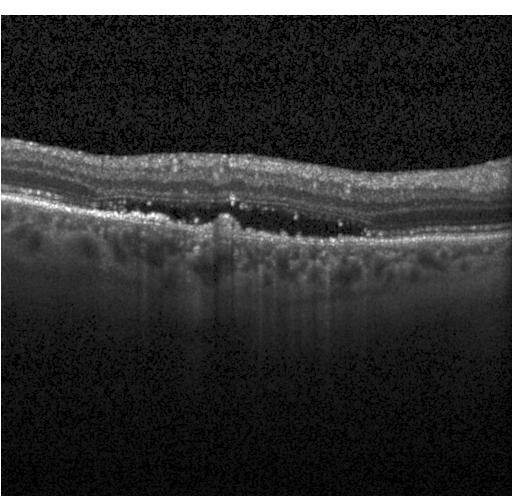 OCT B-scan · instrument: Heidelberg Spectralis.
Assessment: a choroidal neovascular membrane.